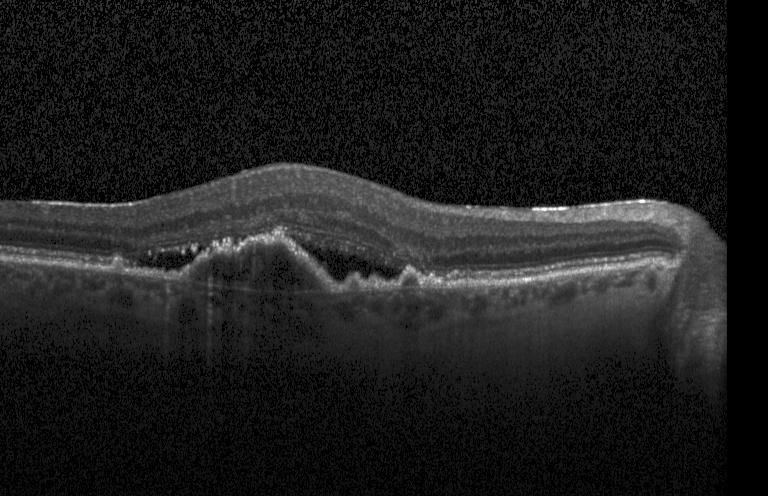
Optical coherence tomography B-scan.
Diagnosis: choroidal neovascularization (CNV).